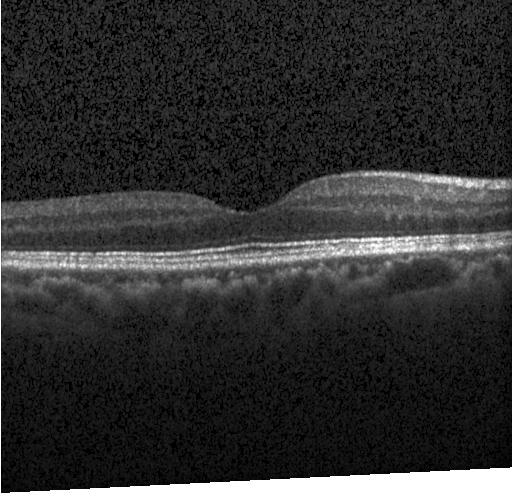

Centered on the fovea; OCT B-scan. This B-scan demonstrates no CNV, no DME, and no drusen.